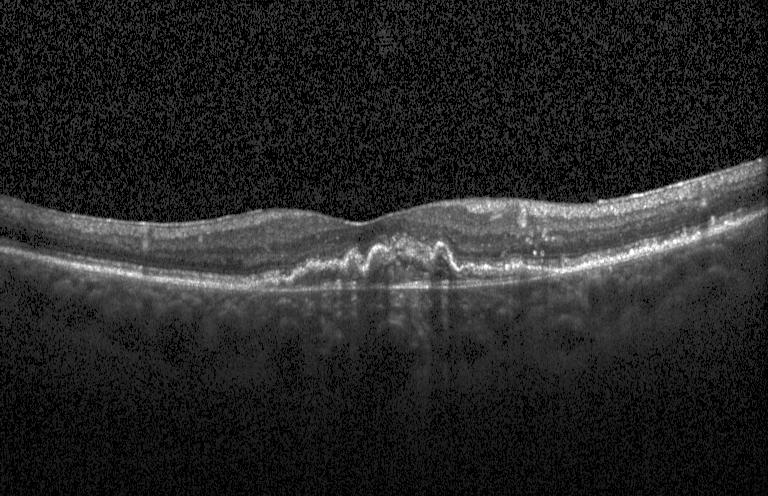

Retinal OCT cross-section, instrument: Heidelberg Spectralis
OCT finding: choroidal neovascularization (CNV).